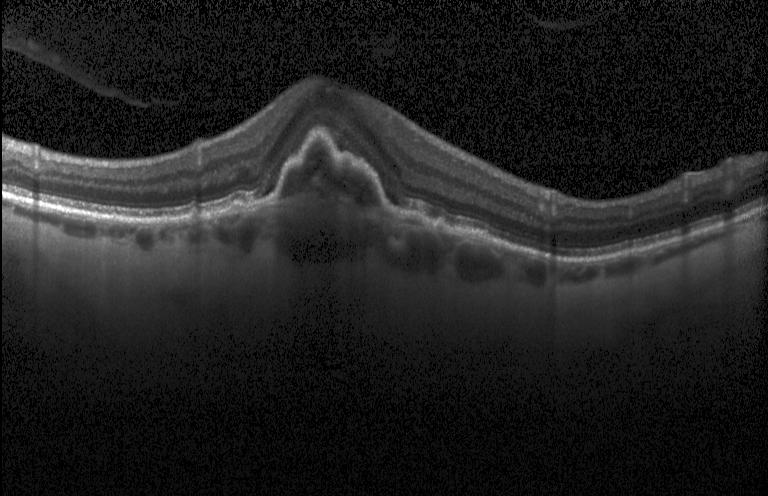

Assessment: a choroidal neovascular membrane.